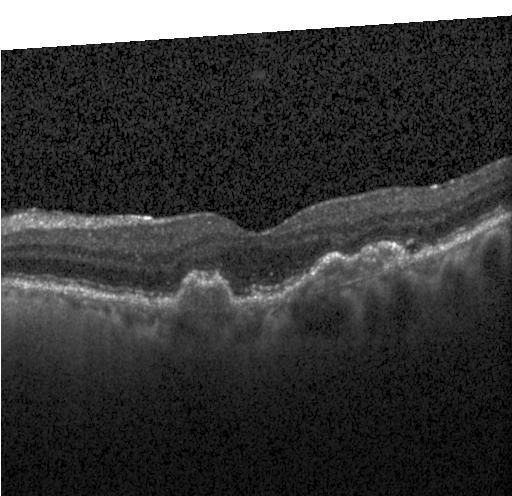 Spectral-domain optical coherence tomography · centered on the fovea · OCT B-scan.
Finding: a choroidal neovascular membrane.